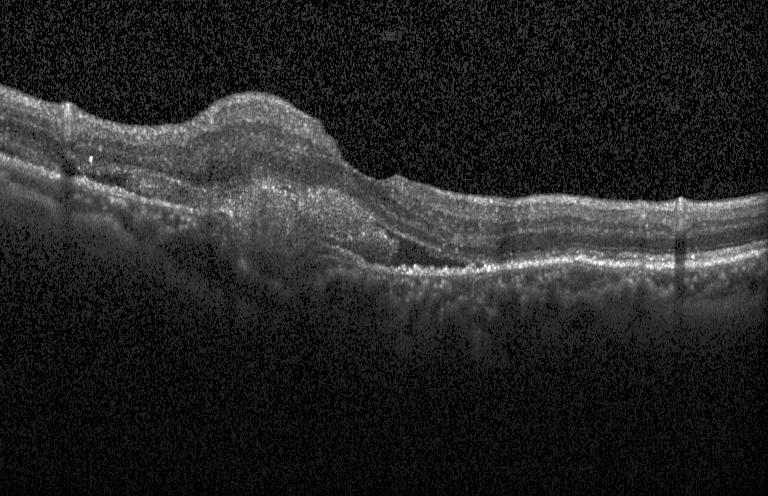 Retinal OCT cross-section — Finding: CNV.